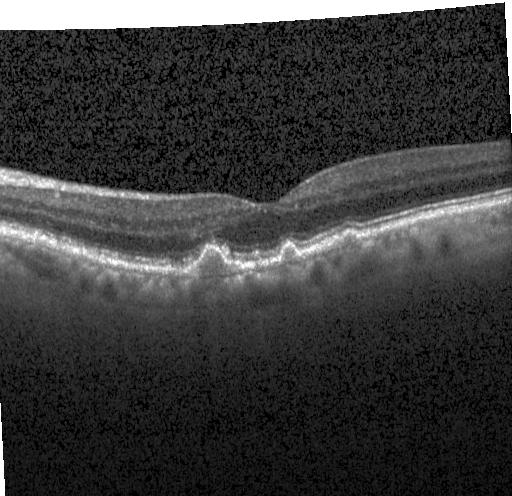

OCT scan showing drusen.